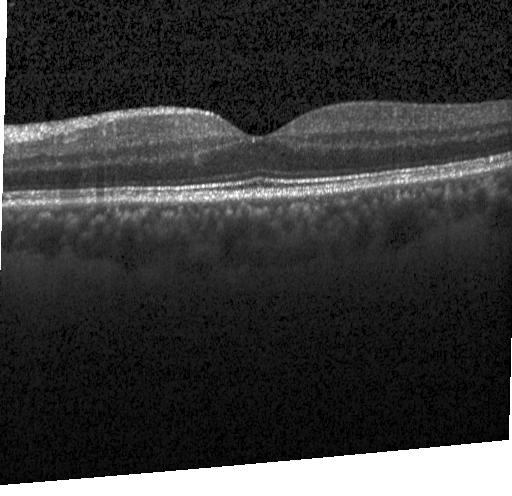 Retinal OCT cross-section. Horizontal scan through the fovea
The scan shows no choroidal neovascularization, diabetic macular edema, or drusen.